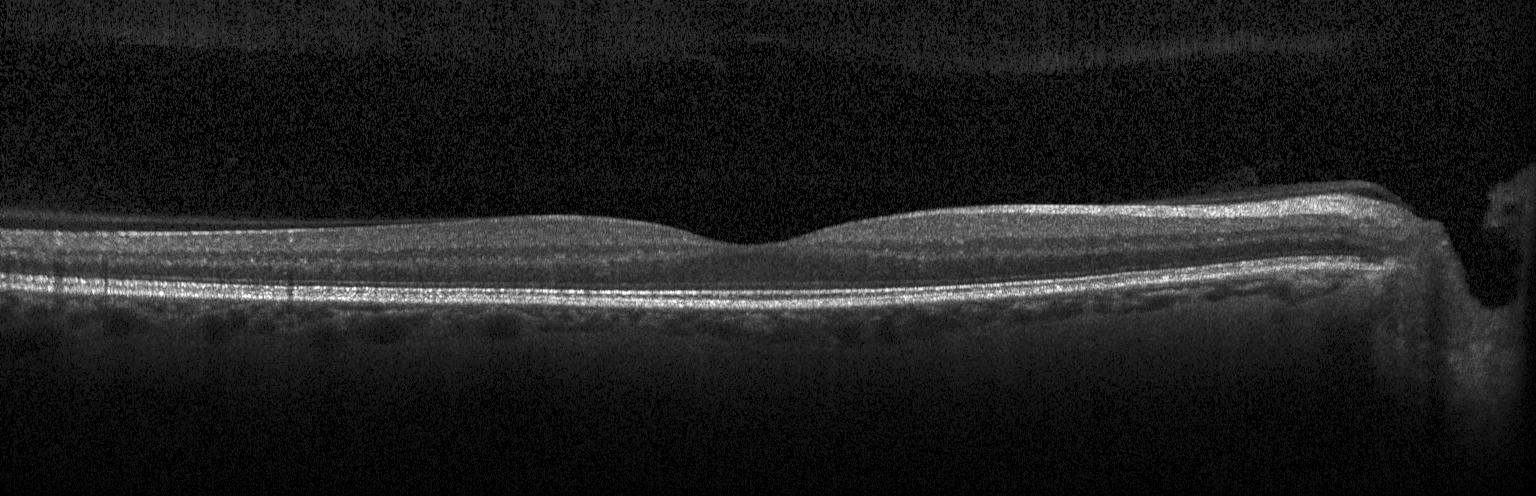
Optical coherence tomography scan — Assessment: no choroidal neovascularization, no diabetic macular edema, and no drusen.